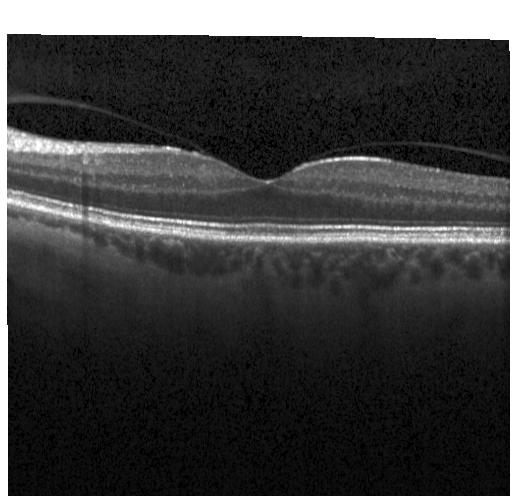

Retinal OCT B-scan, macular scan
Diagnosis: no choroidal neovascularization, diabetic macular edema, or drusen.